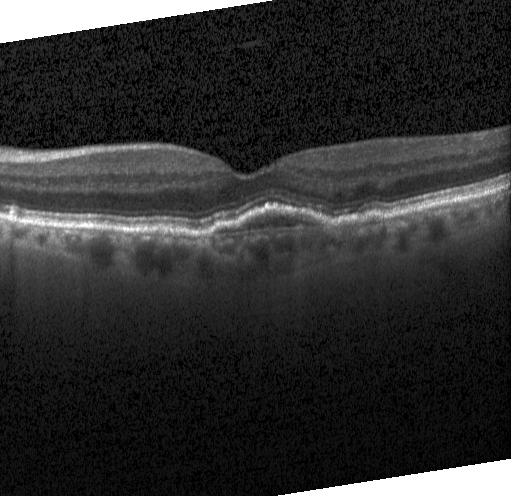

Optical coherence tomography B-scan; macular scan
The scan shows CNV.